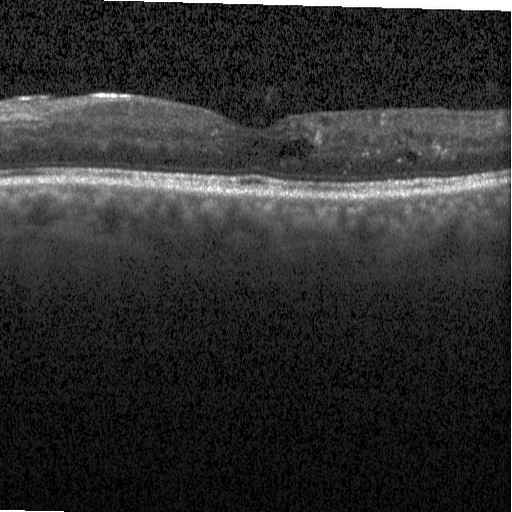

Diagnosis: diabetic macular edema.